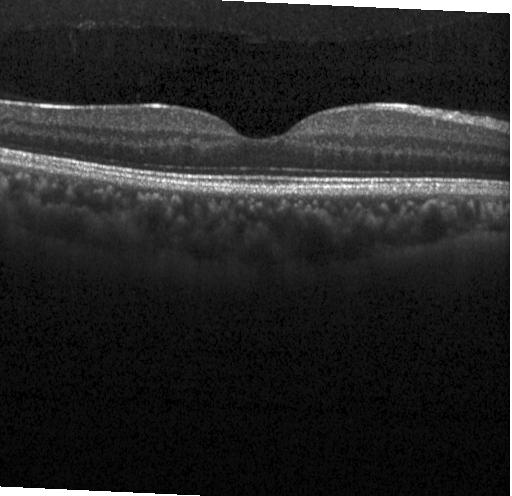 Impression: neither choroidal neovascularization, diabetic macular edema, nor drusen.